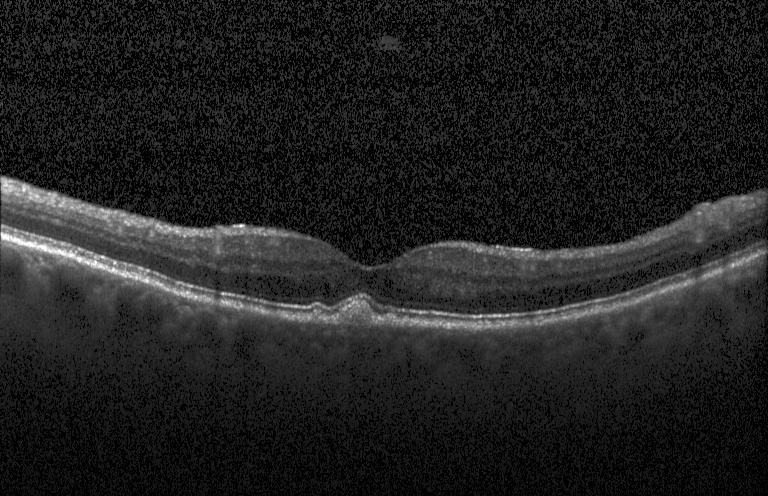
Optical coherence tomography scan. Macular OCT: sub-RPE drusenoid deposits.